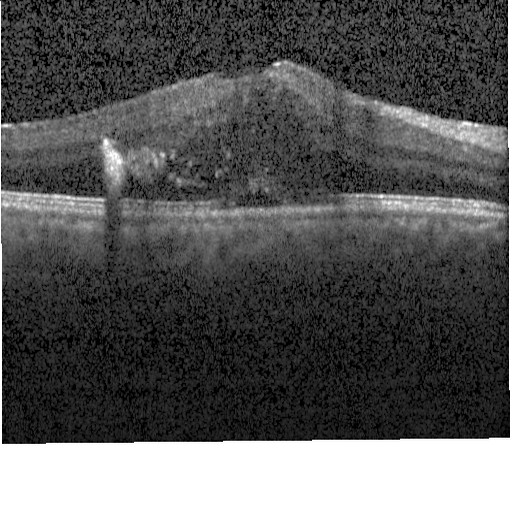
Fovea-centered · spectral-domain OCT · Heidelberg Spectralis OCT system · OCT B-scan.
Impression: diabetic macular edema (DME).